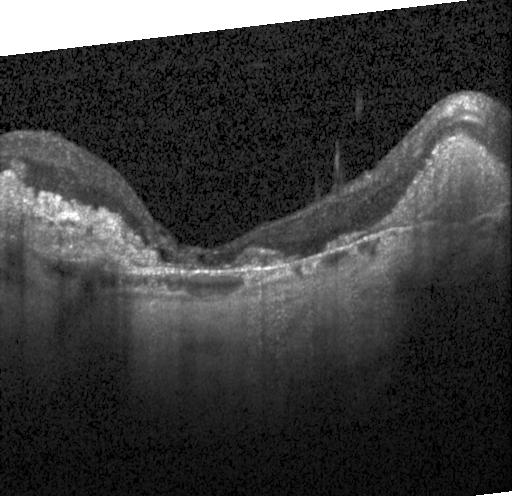

Centered on the fovea. Retinal OCT cross-section. Impression: a choroidal neovascular membrane.